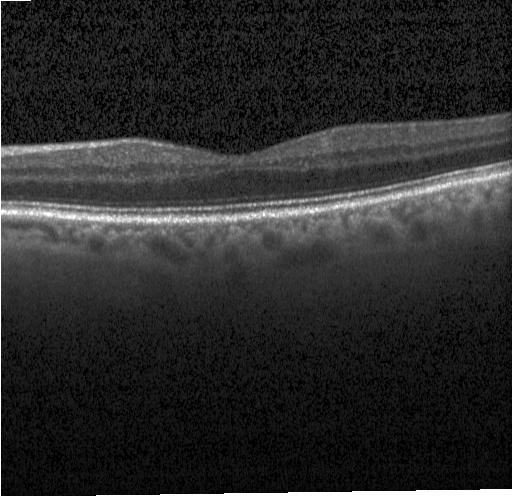

Centered on the fovea, acquired on a Heidelberg Spectralis, retinal OCT B-scan, spectral-domain OCT.
Macular OCT: no evidence of choroidal neovascularization, diabetic macular edema, or drusen.